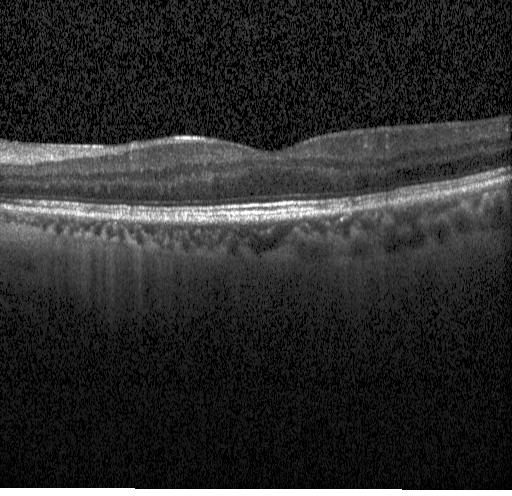
Retinal OCT B-scan · horizontal scan through the fovea.
No choroidal neovascularization, diabetic macular edema, or drusen.